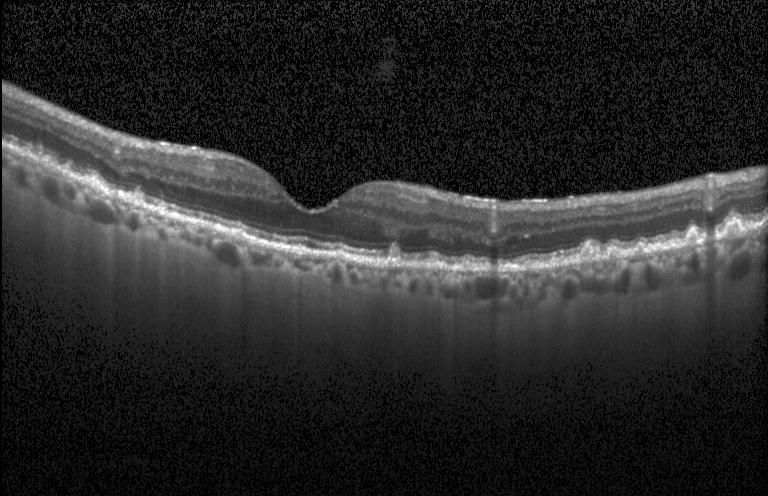

Optical coherence tomography B-scan.
Diagnosis: sub-RPE drusenoid deposits.